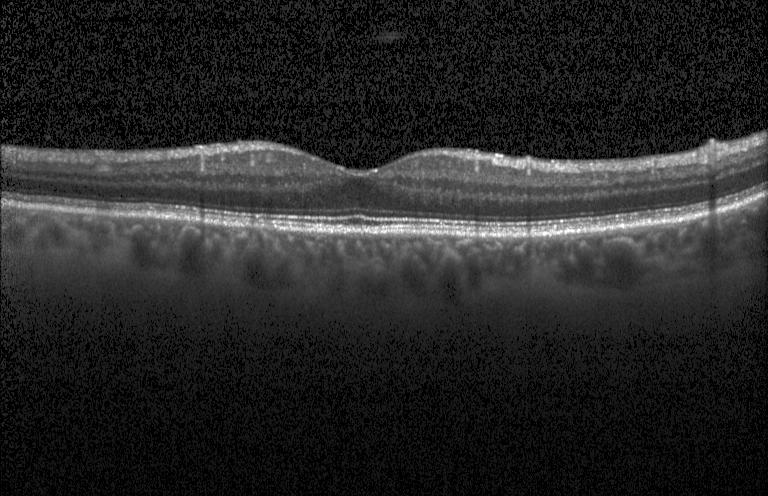

Retinal OCT cross-section, SD-OCT, horizontal scan through the fovea, acquired on a Heidelberg Spectralis.
Impression: neither CNV, DME, nor drusen.